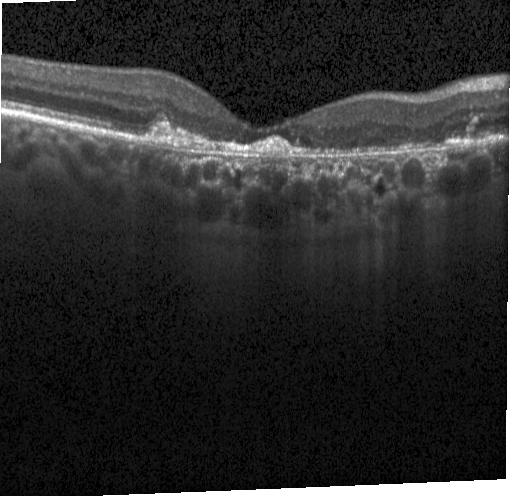
Finding: a choroidal neovascular membrane.